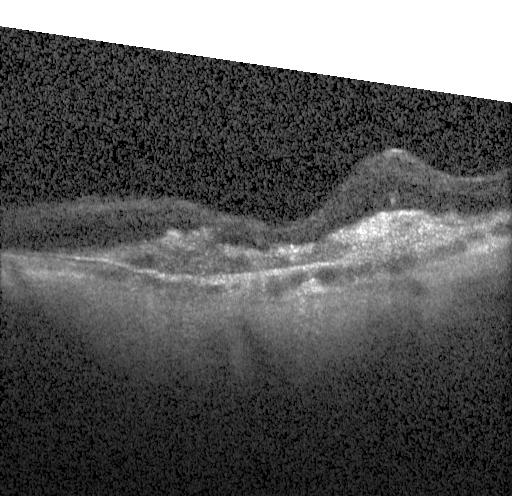

Macular OCT: a choroidal neovascular membrane.